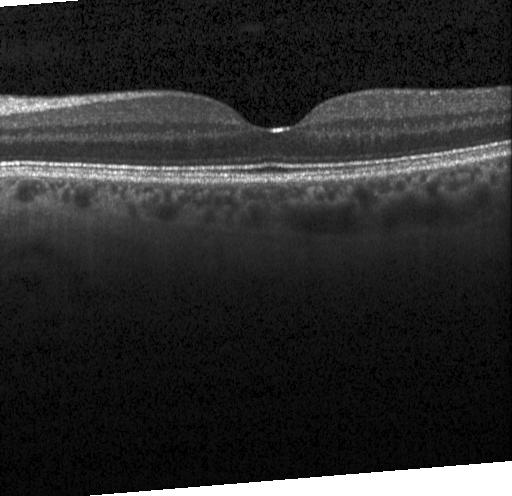 Centered on the fovea, OCT line scan, acquired on a Heidelberg Spectralis — Finding: no CNV, DME, or drusen.